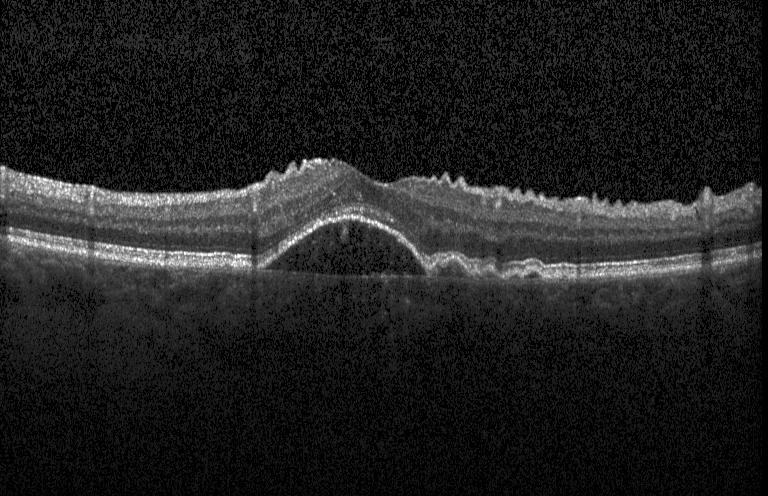

SD-OCT; through the macula; retinal OCT cross-section; Heidelberg Spectralis OCT system
This B-scan demonstrates choroidal neovascularization.